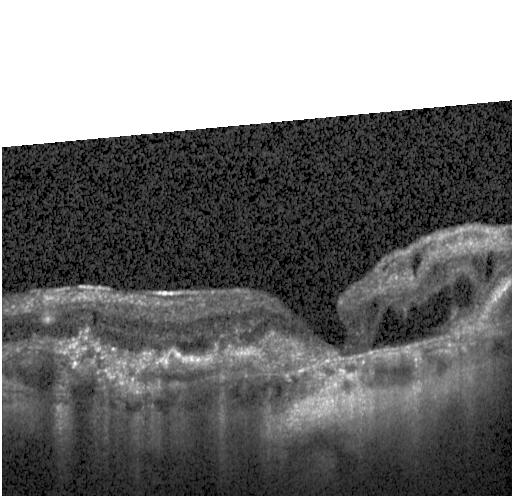

Impression: CNV.